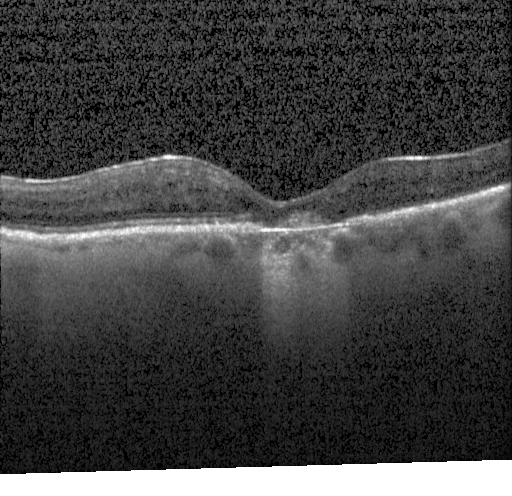 OCT line scan, spectral-domain optical coherence tomography. Assessment: a choroidal neovascular membrane.